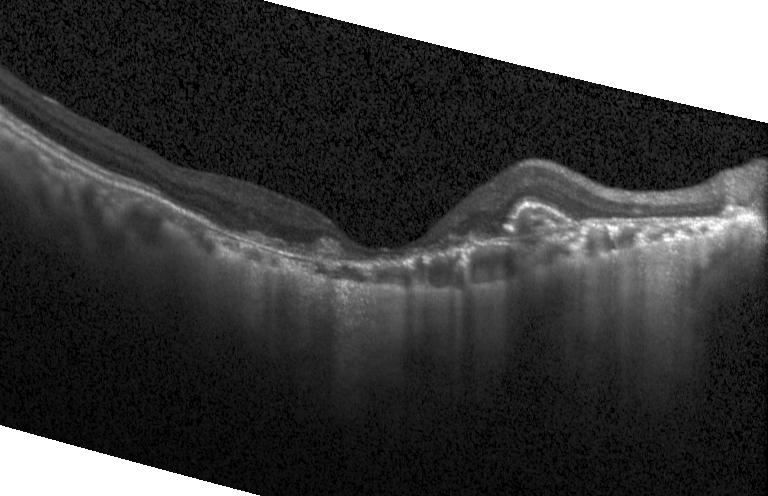
OCT finding: a choroidal neovascular membrane.